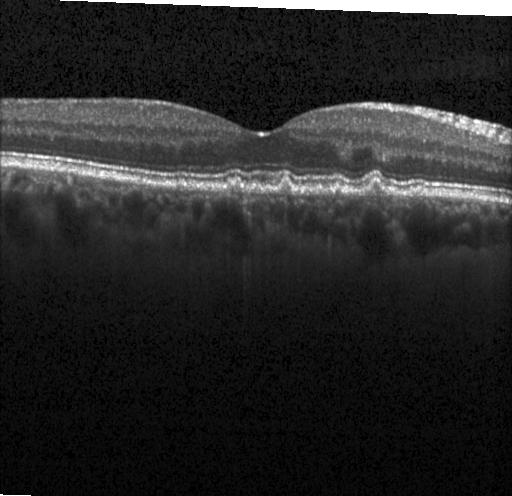

This B-scan demonstrates drusen.